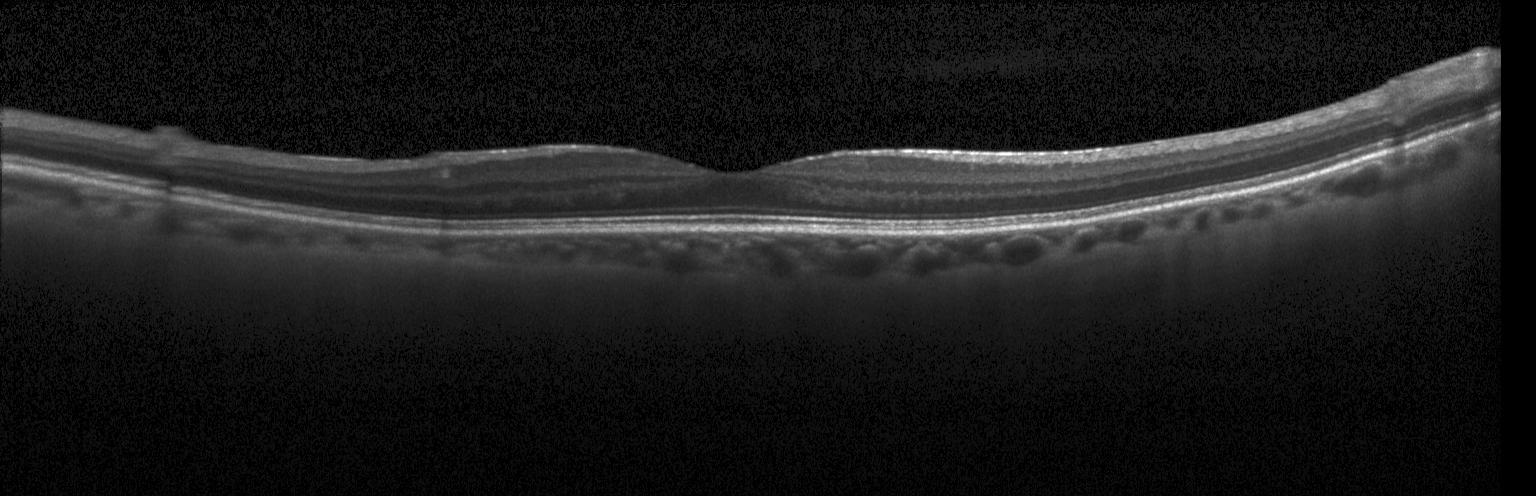 Through the macula · optical coherence tomography B-scan.
Macular OCT: neither CNV, DME, nor drusen.